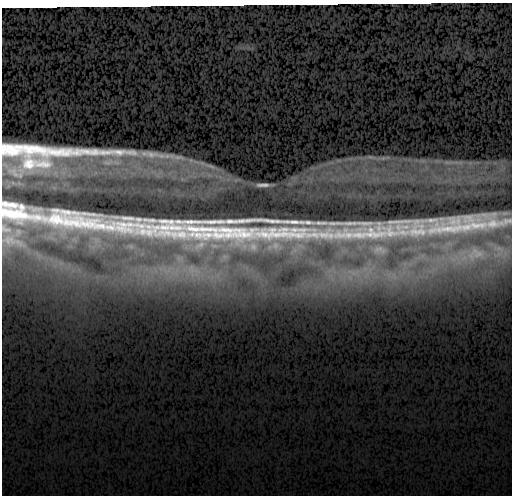
SD-OCT, retinal OCT B-scan, centered on the fovea — No choroidal neovascularization, diabetic macular edema, or drusen.